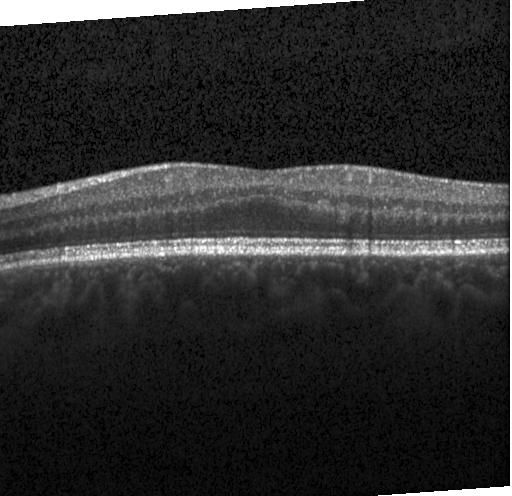 Optical coherence tomography scan — Finding: no choroidal neovascularization, no diabetic macular edema, and no drusen.